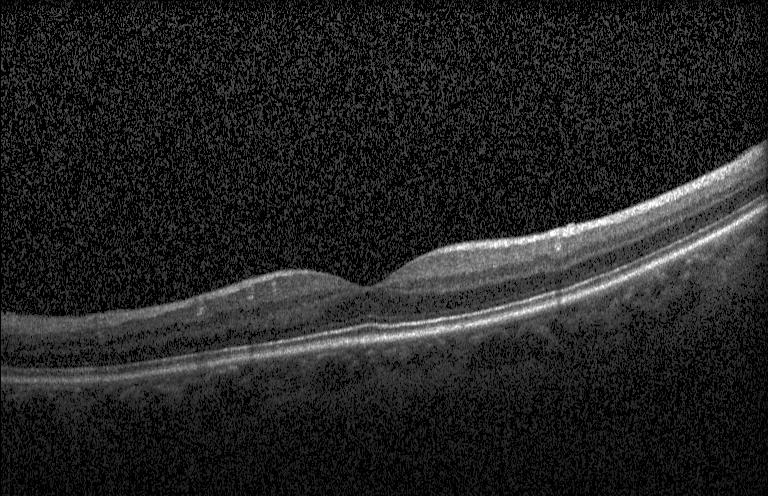
Spectral-domain optical coherence tomography, retinal OCT cross-section, macular scan
Finding: no choroidal neovascularization, diabetic macular edema, or drusen.